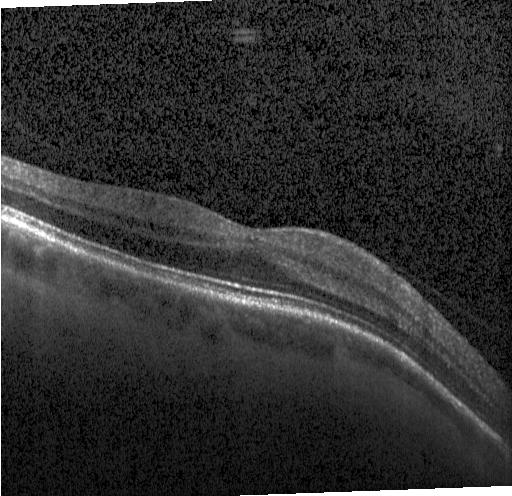 Dx: neither CNV, DME, nor drusen.